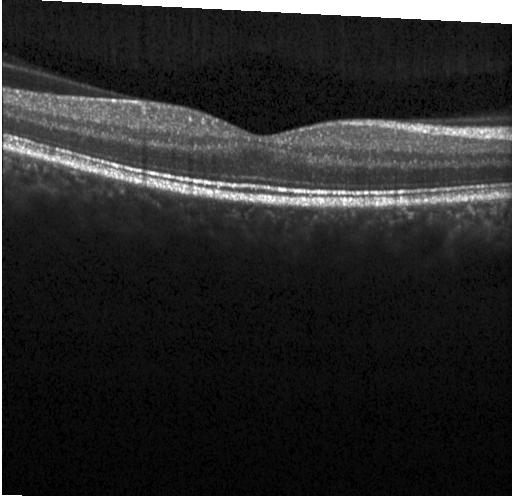 Impression: no choroidal neovascularization, diabetic macular edema, or drusen.